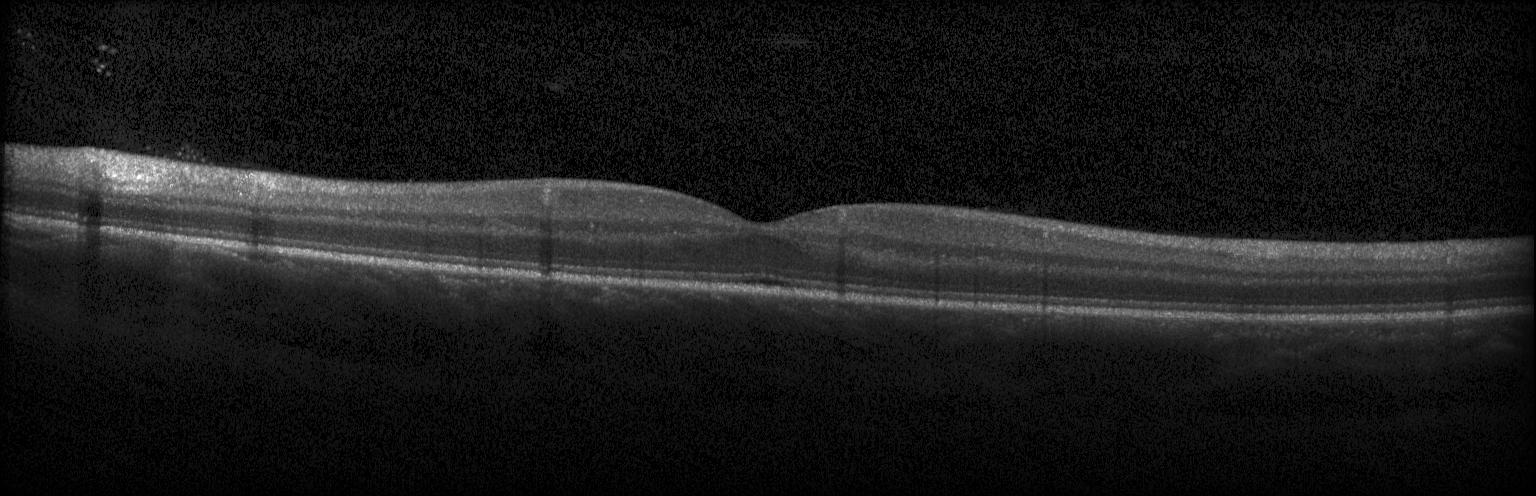

OCT B-scan showing no evidence of choroidal neovascularization, diabetic macular edema, or drusen.